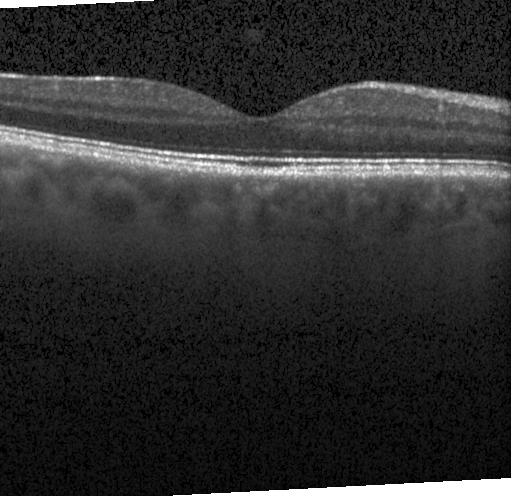 OCT line scan. Dx: neither choroidal neovascularization, diabetic macular edema, nor drusen.